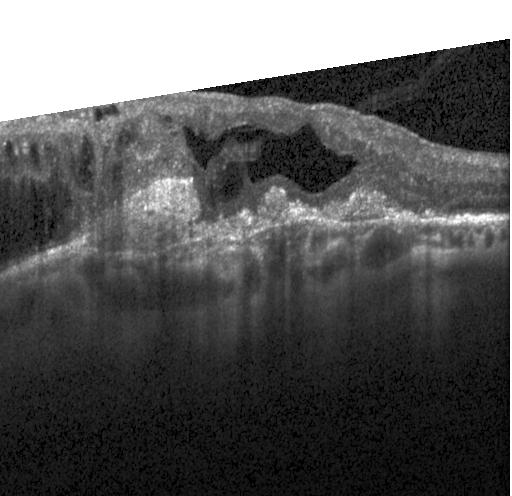 Retinal OCT cross-section, spectral-domain OCT, Heidelberg Spectralis OCT system.
Impression: a choroidal neovascular membrane.